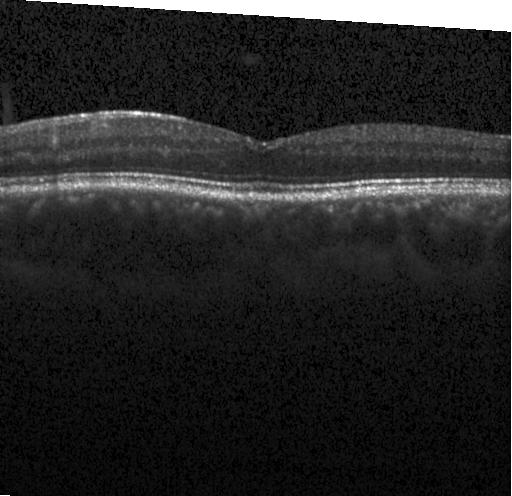 Impression: no evidence of choroidal neovascularization, diabetic macular edema, or drusen.